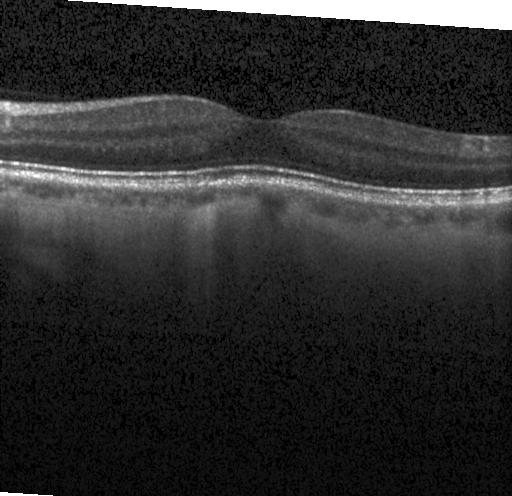
Macular OCT demonstrating no choroidal neovascularization, no diabetic macular edema, and no drusen.